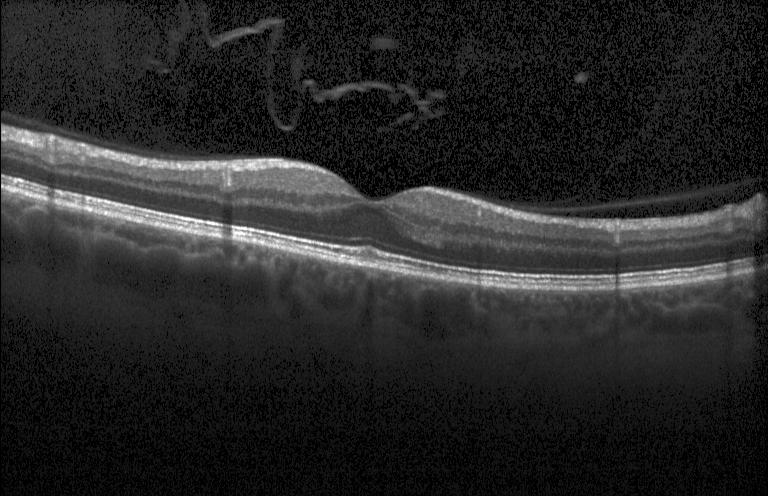 Optical coherence tomography B-scan — Macular OCT: no evidence of choroidal neovascularization, diabetic macular edema, or drusen.